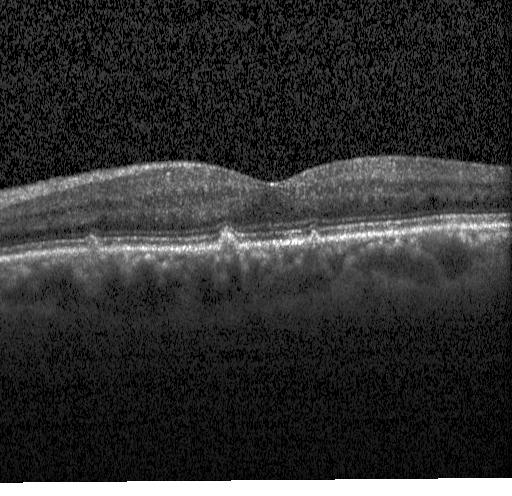 Finding: sub-RPE drusenoid deposits.